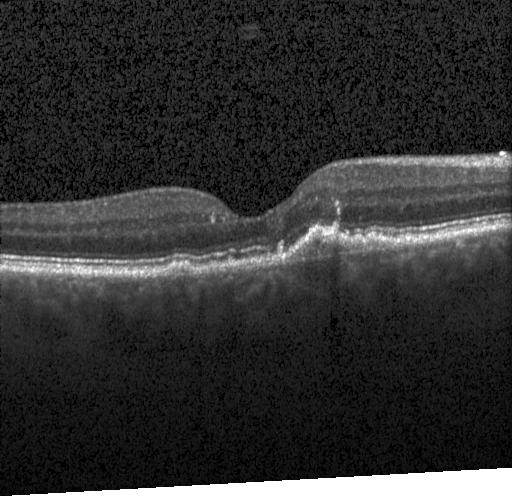 Optical coherence tomography B-scan · through the macula · SD-OCT · instrument: Heidelberg Spectralis. Impression: a choroidal neovascular membrane.